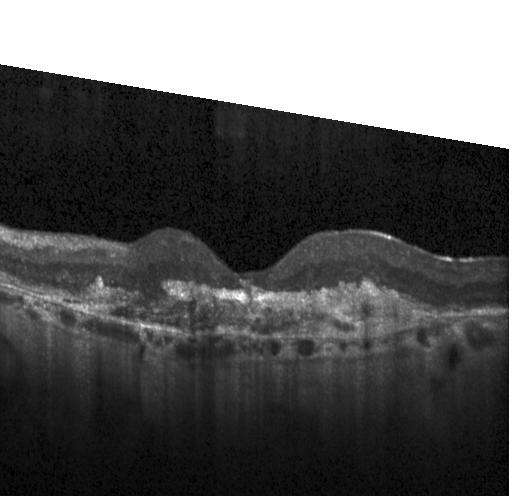

Impression: choroidal neovascularization (CNV).